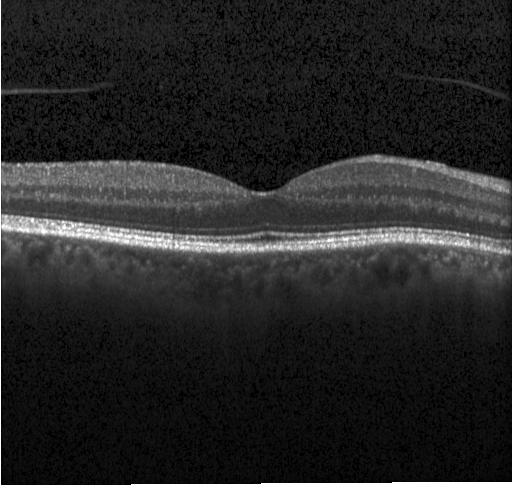
Through the macula. Instrument: Heidelberg Spectralis. OCT line scan. Spectral-domain optical coherence tomography
Finding: neither choroidal neovascularization, diabetic macular edema, nor drusen.